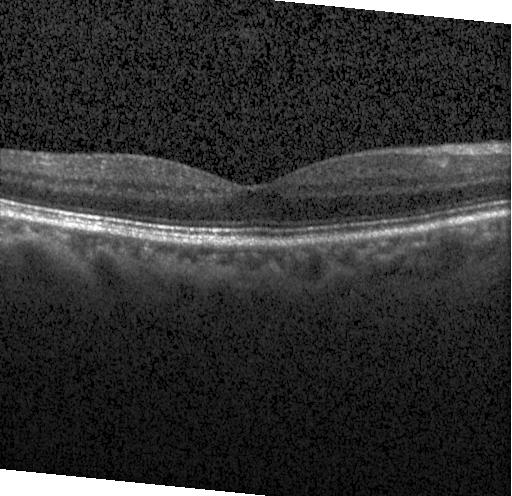

No choroidal neovascularization, no diabetic macular edema, and no drusen.